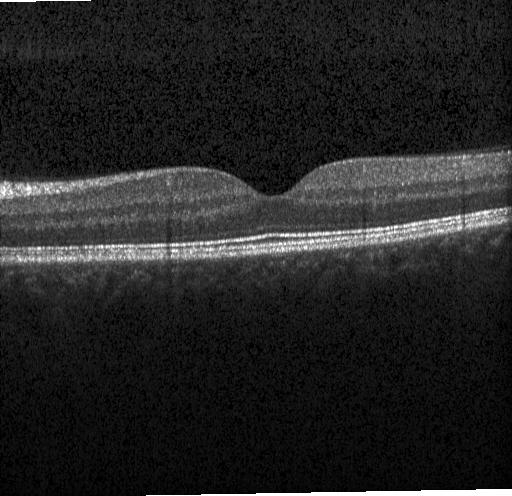
Optical coherence tomography scan — Assessment: neither CNV, DME, nor drusen.